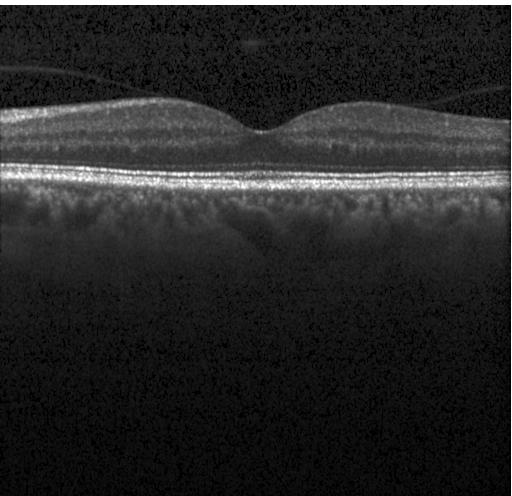 Heidelberg Spectralis OCT system, horizontal scan through the fovea, SD-OCT, retinal OCT cross-section
No choroidal neovascularization, diabetic macular edema, or drusen.